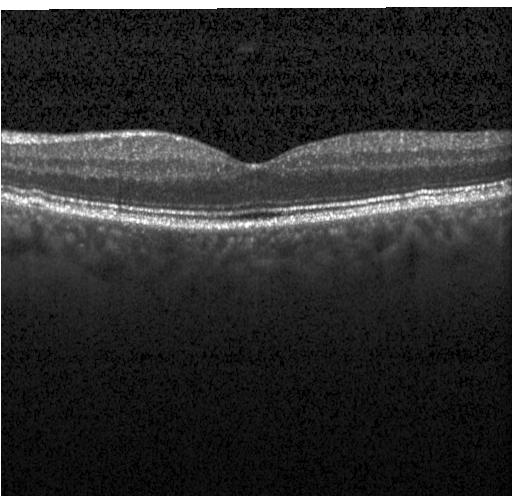 SD-OCT; OCT B-scan; Heidelberg Spectralis OCT system; horizontal scan through the fovea
Finding: neither CNV, DME, nor drusen.